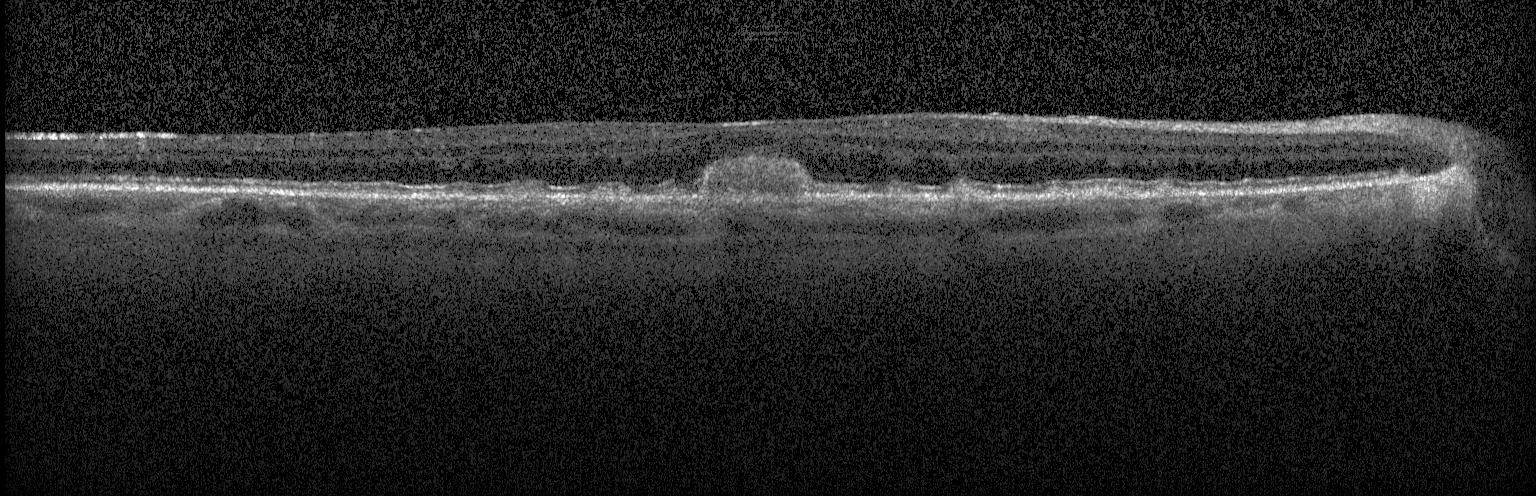 Through the macula · retinal OCT cross-section. This B-scan demonstrates choroidal neovascularization.